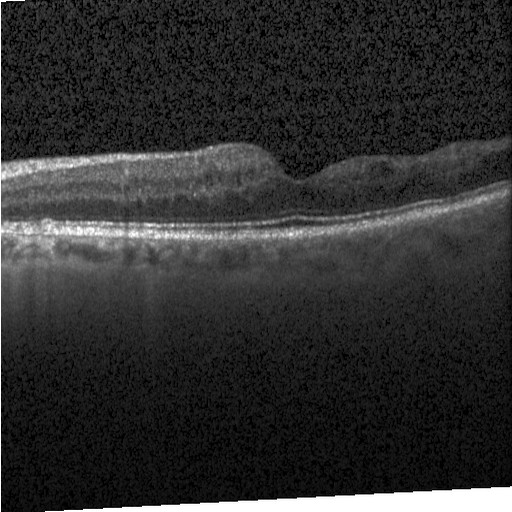
Assessment: diabetic macular edema (DME).